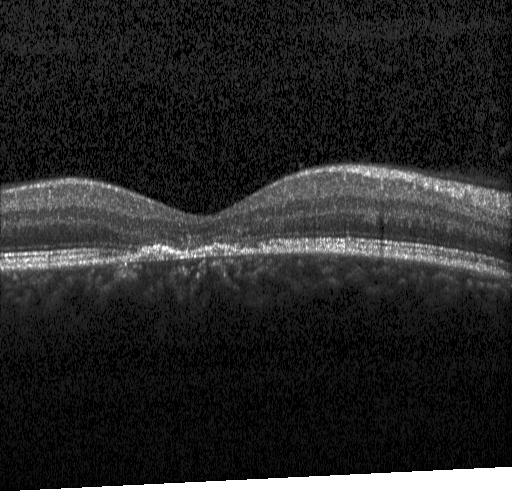 Horizontal scan through the fovea · instrument: Heidelberg Spectralis · retinal OCT cross-section.
Assessment: a choroidal neovascular membrane.